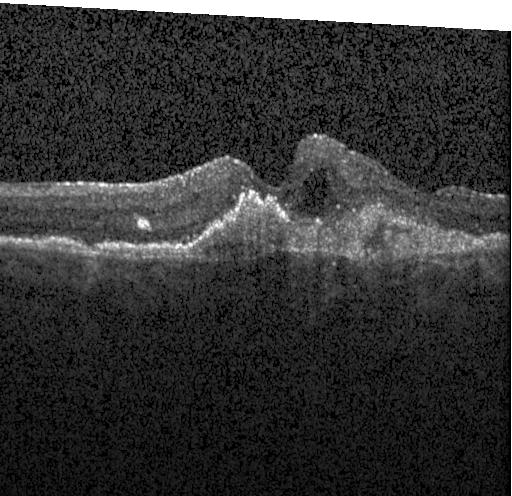
Retinal OCT cross-section, through the macula, spectral-domain optical coherence tomography. Impression: a choroidal neovascular membrane.